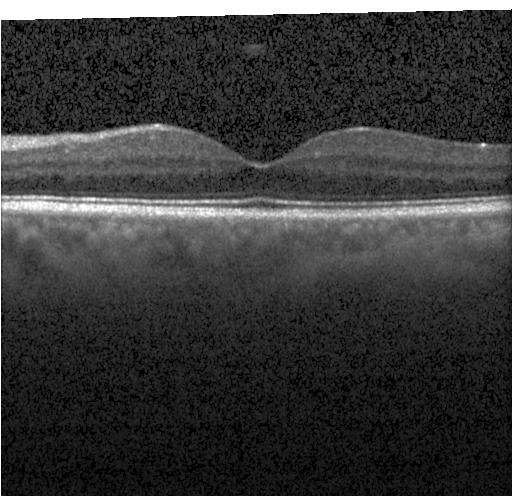 Macular OCT: no choroidal neovascularization, diabetic macular edema, or drusen.